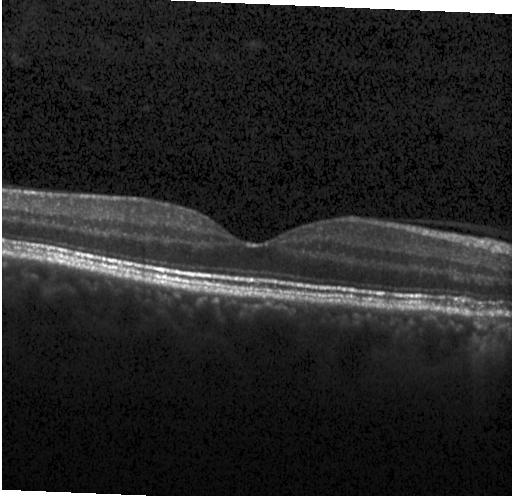 Optical coherence tomography scan. Spectral-domain optical coherence tomography
Assessment: no choroidal neovascularization, diabetic macular edema, or drusen.